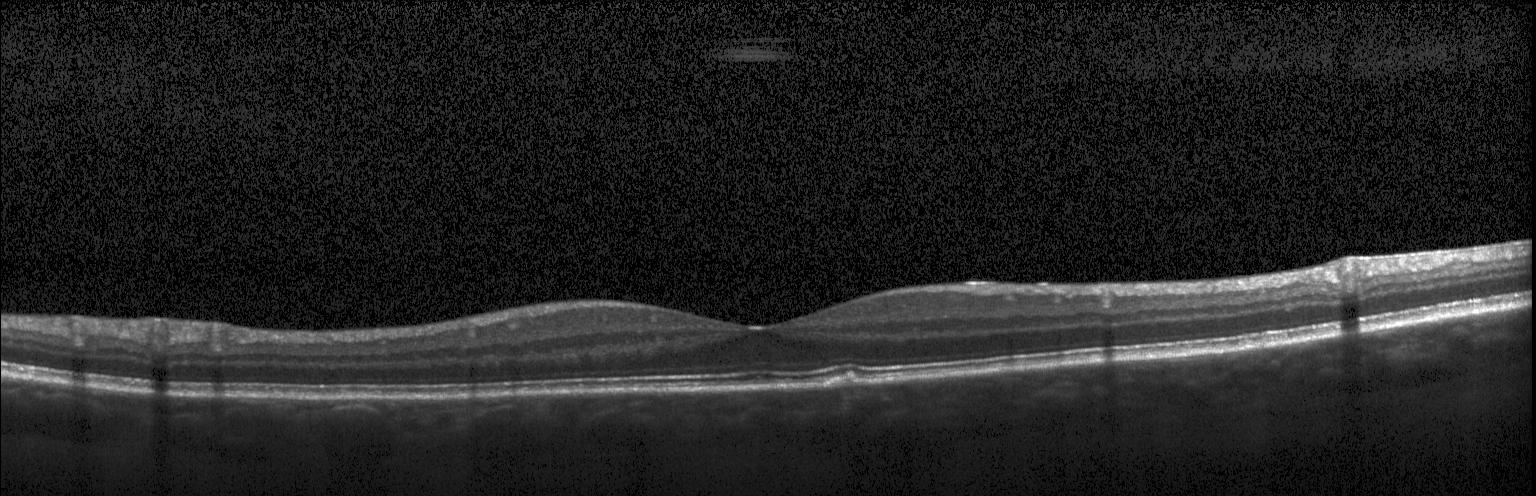 Impression: multiple drusen.